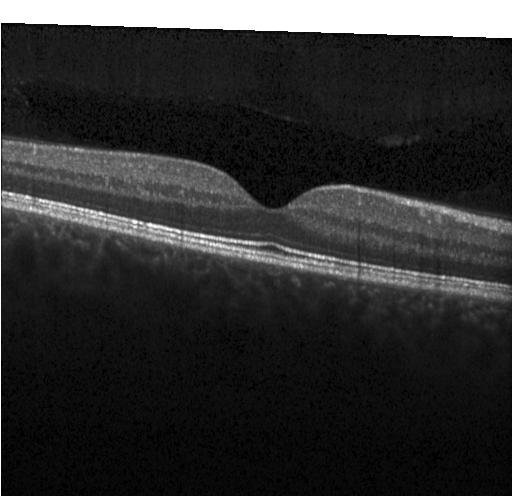

OCT B-scan showing no CNV, DME, or drusen.